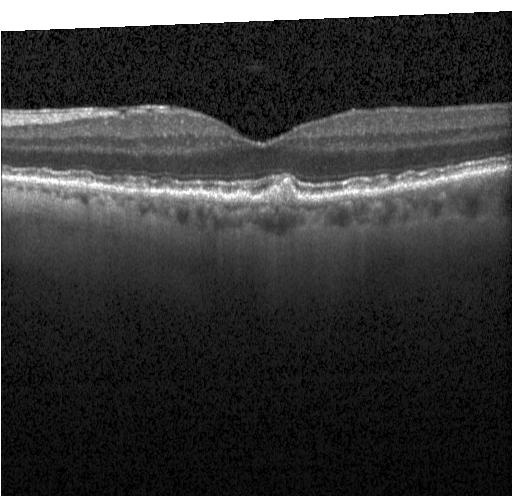

Retinal OCT cross-section · Heidelberg Spectralis OCT system.
Assessment: drusen.